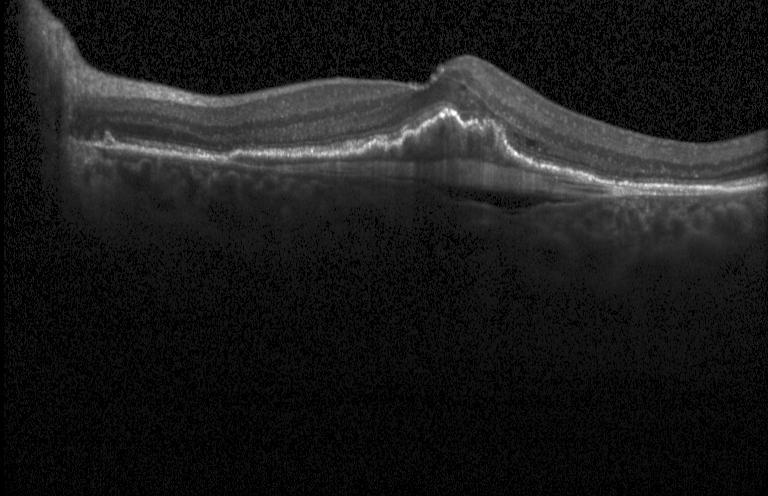
Spectral-domain OCT. OCT B-scan. Through the macula. Heidelberg Spectralis OCT system
Diagnosis: choroidal neovascularization (CNV).